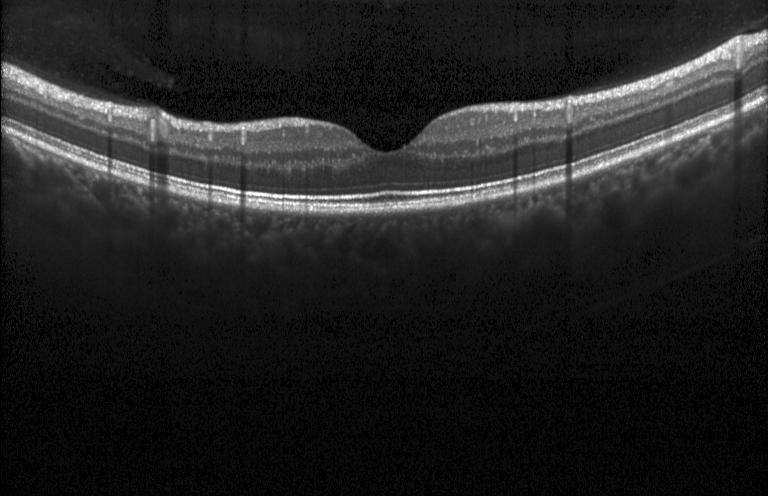 OCT B-scan. Assessment: no choroidal neovascularization, no diabetic macular edema, and no drusen.